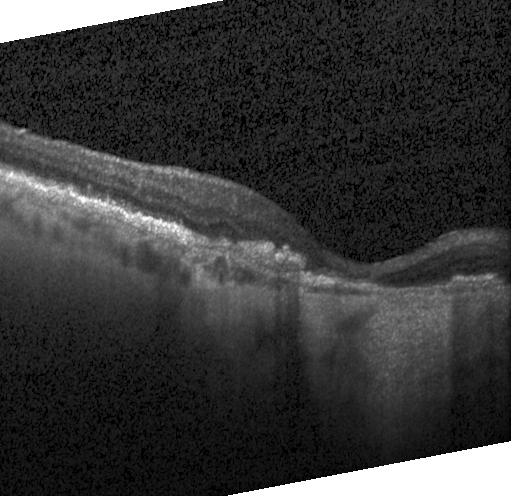
Optical coherence tomography scan, acquired on a Heidelberg Spectralis, spectral-domain optical coherence tomography — CNV.